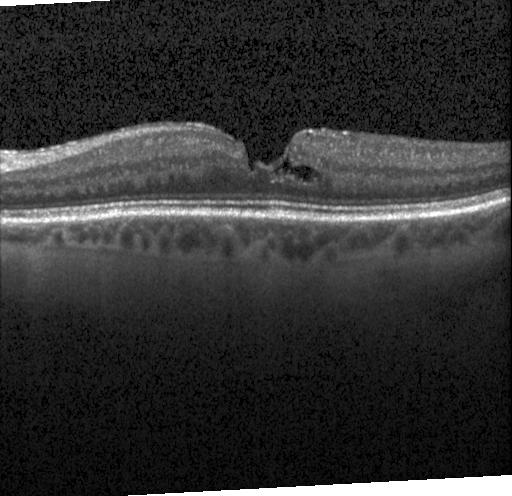
Spectral-domain OCT; OCT line scan. Impression: diabetic macular edema.